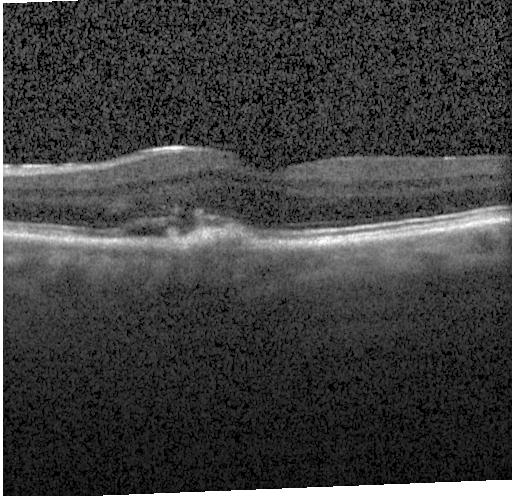

OCT finding: choroidal neovascularization (CNV).